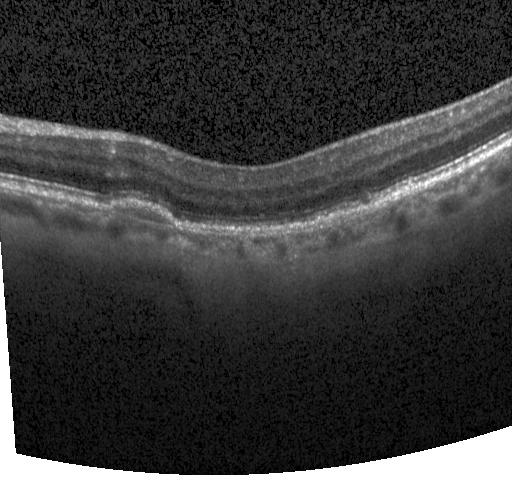 Optical coherence tomography scan, acquired on a Heidelberg Spectralis, spectral-domain optical coherence tomography
Diagnosis: CNV.